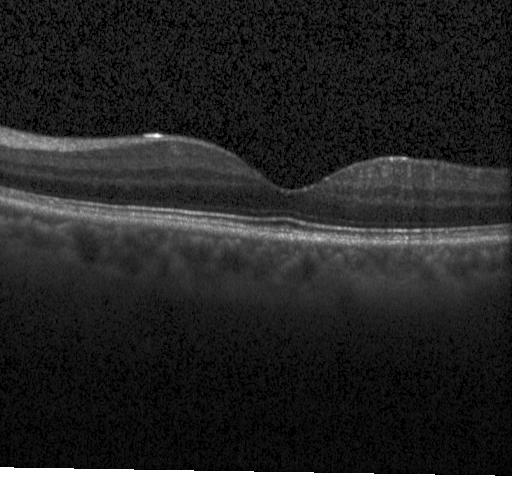
Assessment: neither choroidal neovascularization, diabetic macular edema, nor drusen.